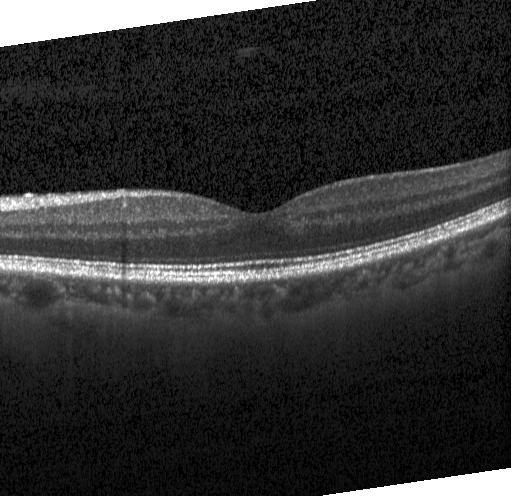
Optical coherence tomography scan; SD-OCT; fovea-centered. Impression: neither choroidal neovascularization, diabetic macular edema, nor drusen.